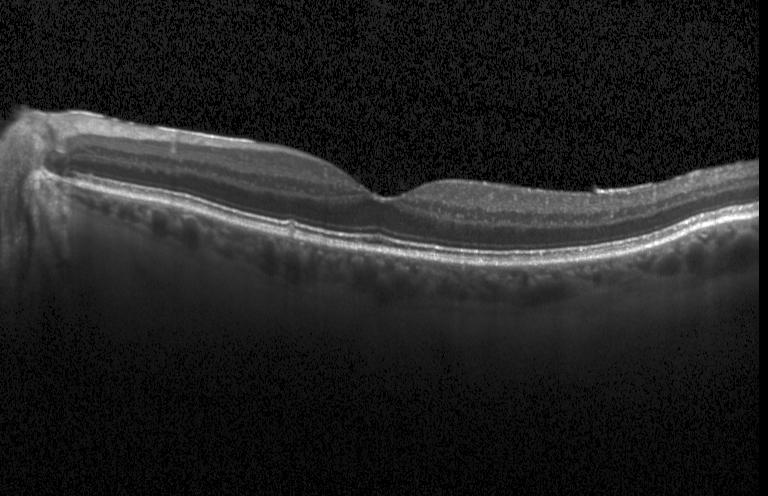

Centered on the fovea · SD-OCT · acquired on a Heidelberg Spectralis · retinal OCT cross-section. Diagnosis: no choroidal neovascularization, diabetic macular edema, or drusen.